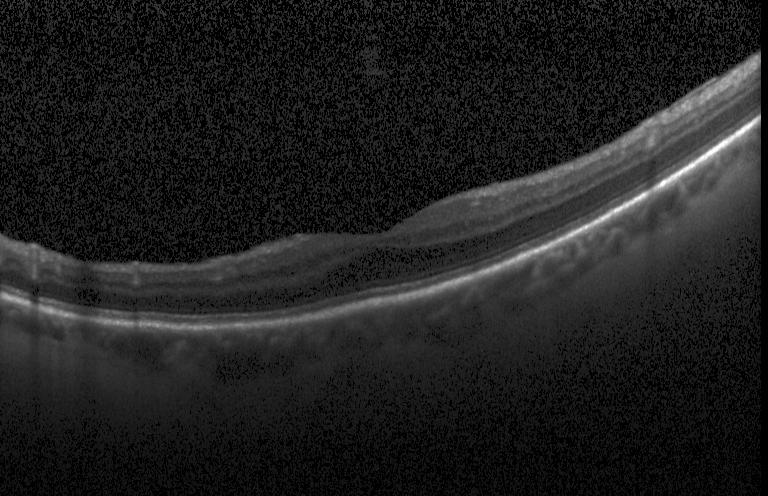 Instrument: Heidelberg Spectralis; spectral-domain OCT; OCT B-scan. Assessment: neither choroidal neovascularization, diabetic macular edema, nor drusen.